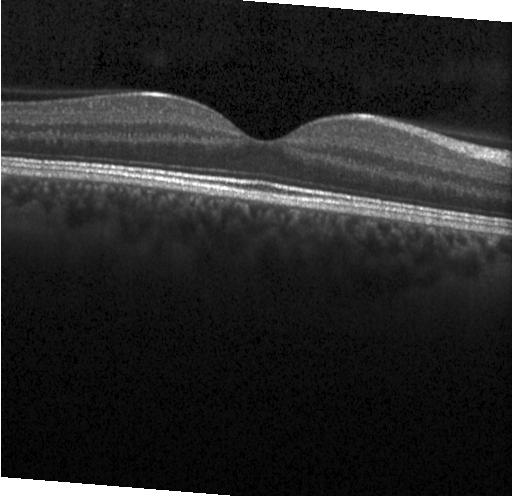 Retinal OCT cross-section · SD-OCT · centered on the fovea · instrument: Heidelberg Spectralis — OCT finding: neither choroidal neovascularization, diabetic macular edema, nor drusen.